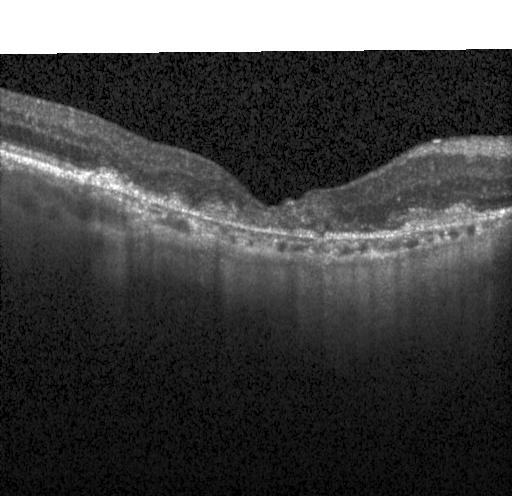
OCT line scan — This B-scan demonstrates a choroidal neovascular membrane.